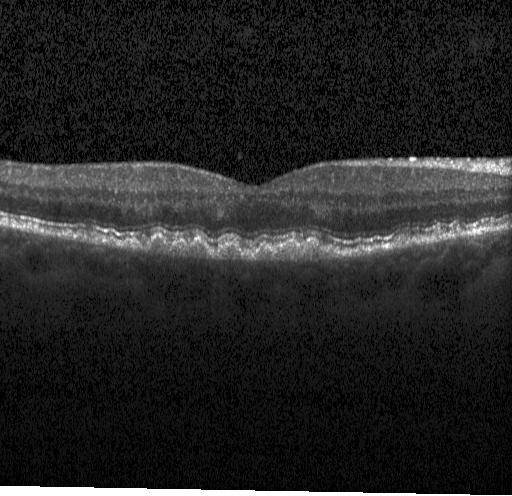 Instrument: Heidelberg Spectralis. Macular scan. Retinal OCT B-scan. Diagnosis: multiple drusen.